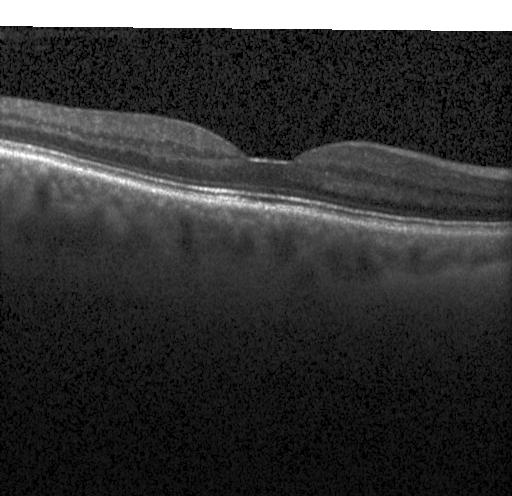
SD-OCT; optical coherence tomography scan. Assessment: neither choroidal neovascularization, diabetic macular edema, nor drusen.